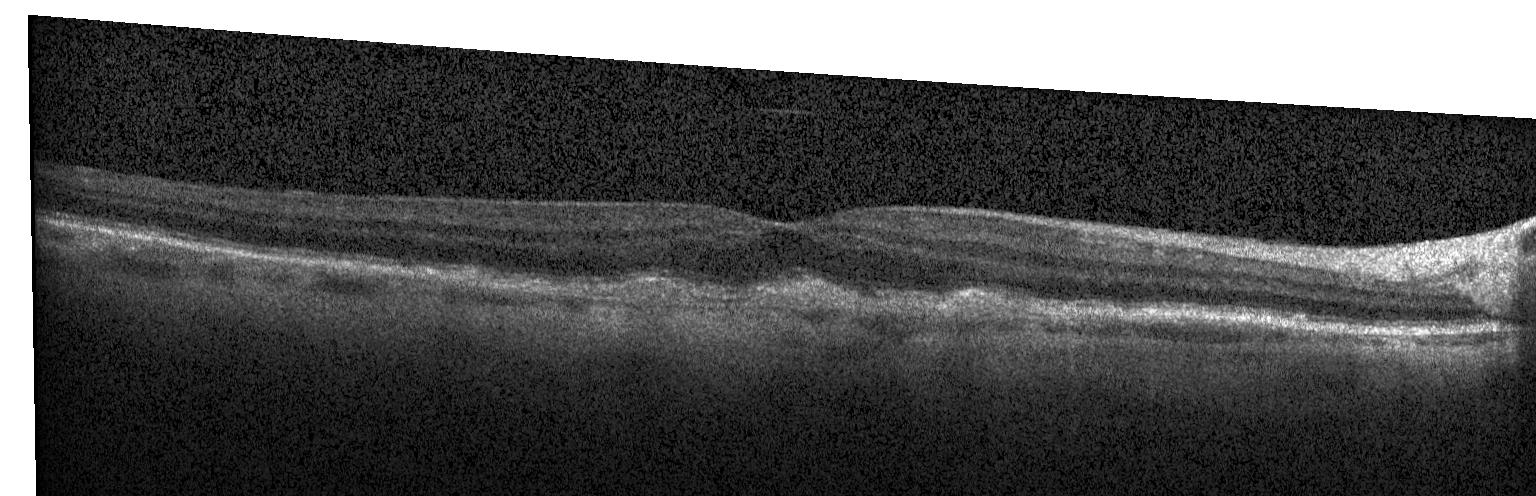 OCT finding: choroidal neovascularization.